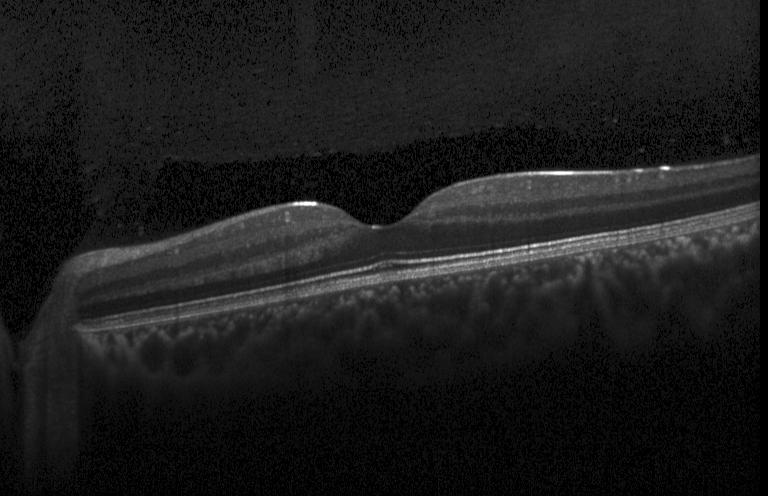
OCT B-scan, fovea-centered, spectral-domain optical coherence tomography. Impression: no CNV, no DME, and no drusen.